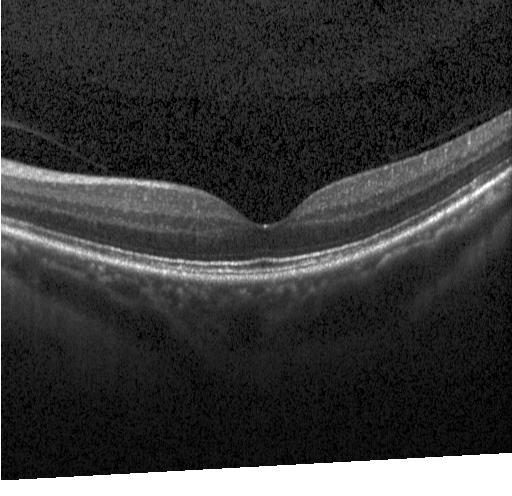
Impression: no choroidal neovascularization, no diabetic macular edema, and no drusen.